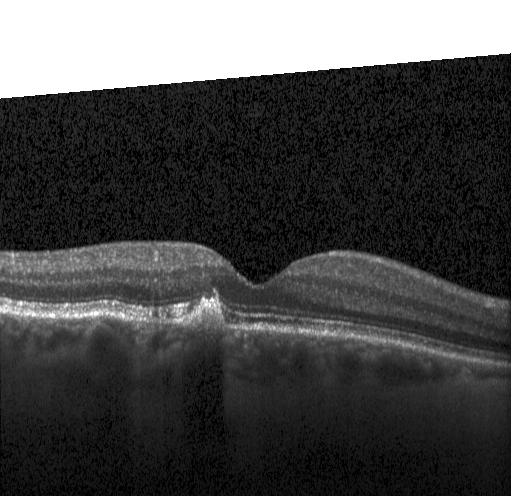
Diagnosis: sub-RPE drusenoid deposits.